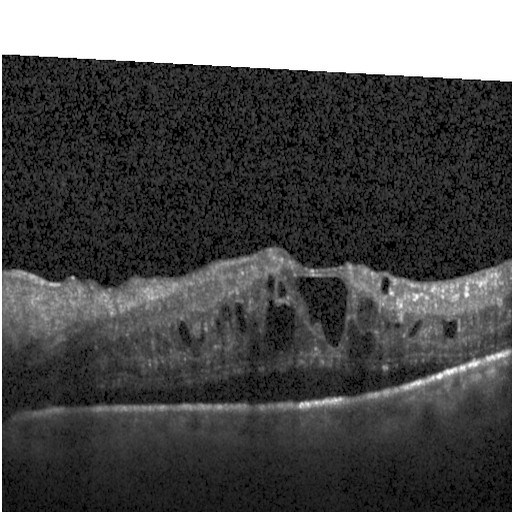
Retinal OCT cross-section. Heidelberg Spectralis OCT system. Spectral-domain optical coherence tomography. Through the macula
OCT finding: diabetic macular edema (DME).